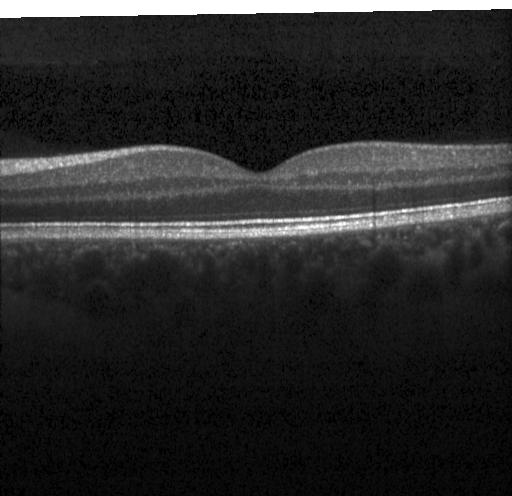 OCT line scan, through the macula, spectral-domain optical coherence tomography, instrument: Heidelberg Spectralis — OCT finding: neither CNV, DME, nor drusen.